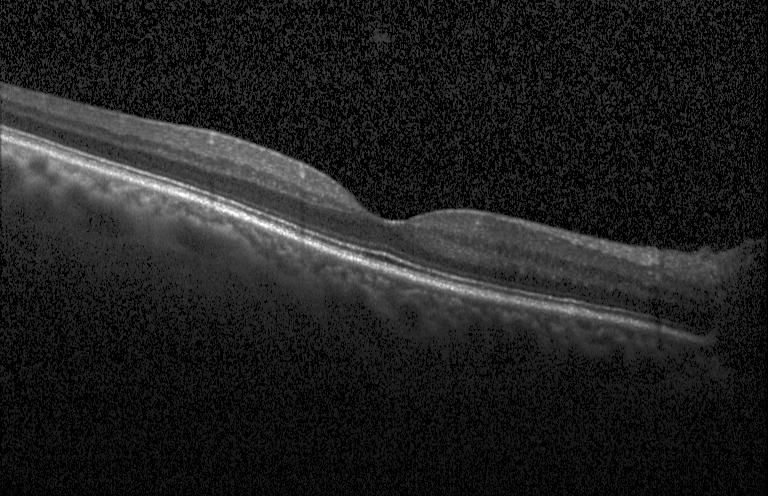

Spectral-domain OCT B-scan: no choroidal neovascularization, no diabetic macular edema, and no drusen.